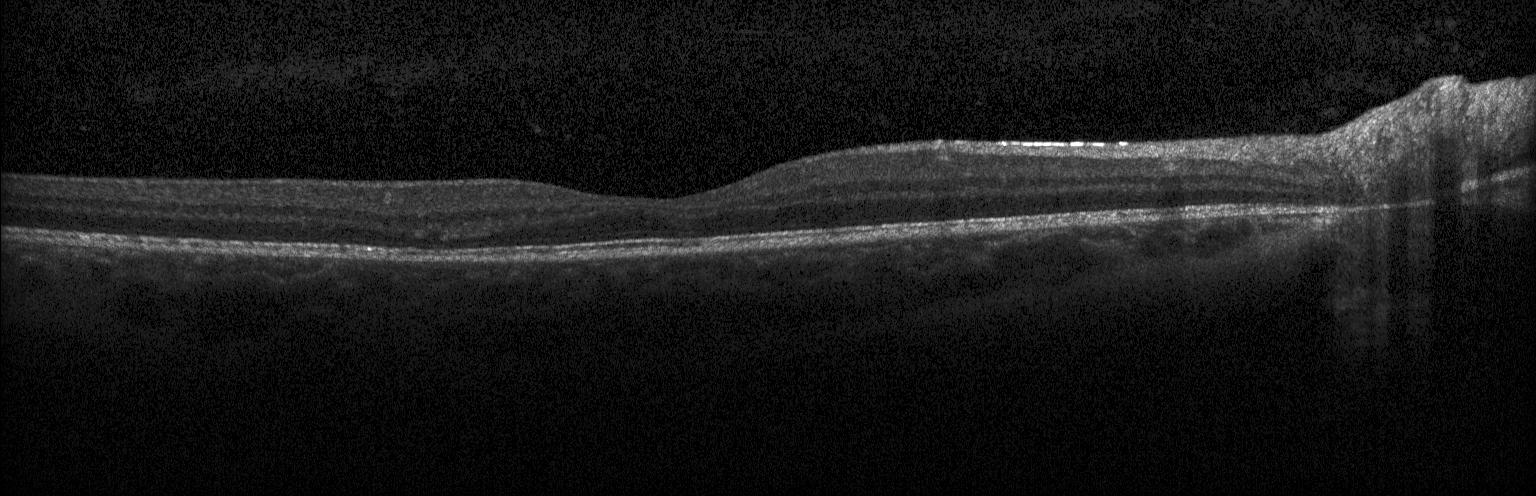

Optical coherence tomography scan; fovea-centered
The scan shows neither choroidal neovascularization, diabetic macular edema, nor drusen.